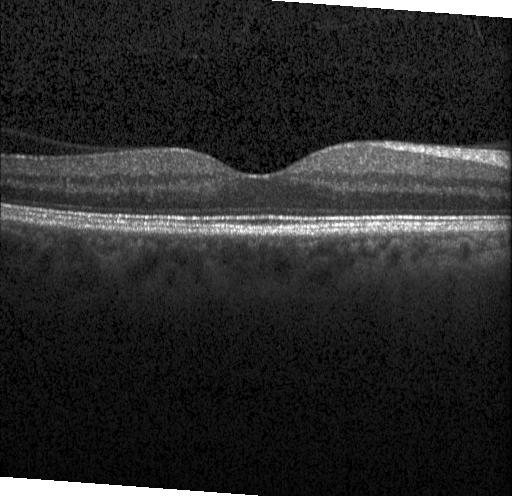

OCT line scan. Diagnosis: neither CNV, DME, nor drusen.